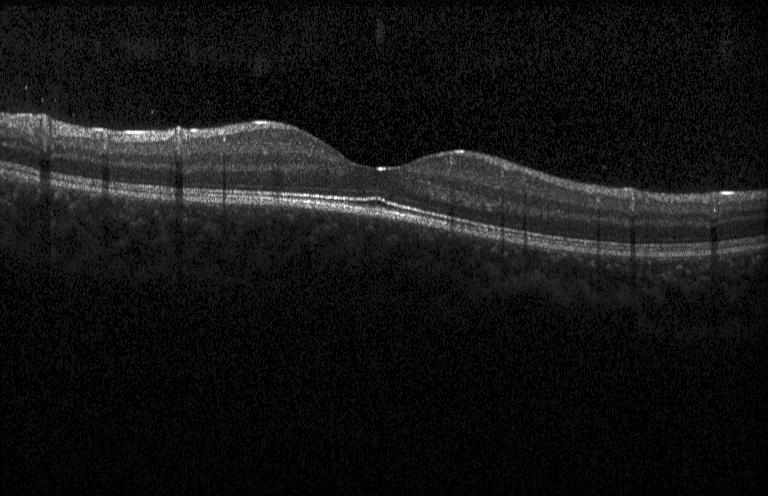

Heidelberg Spectralis · spectral-domain optical coherence tomography · retinal OCT cross-section · through the macula. Diagnosis: no choroidal neovascularization, diabetic macular edema, or drusen.